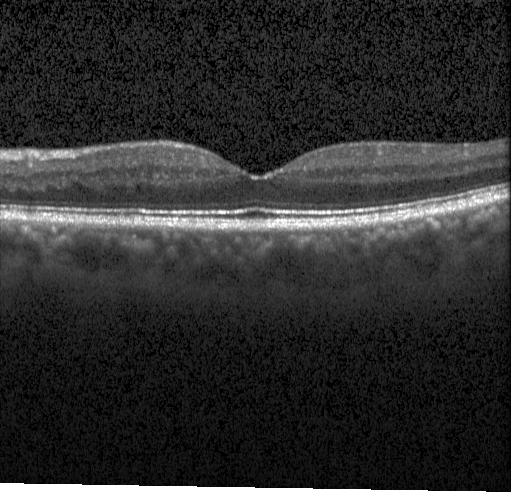

SD-OCT, Heidelberg Spectralis OCT system, through the macula, OCT B-scan
This B-scan demonstrates neither choroidal neovascularization, diabetic macular edema, nor drusen.